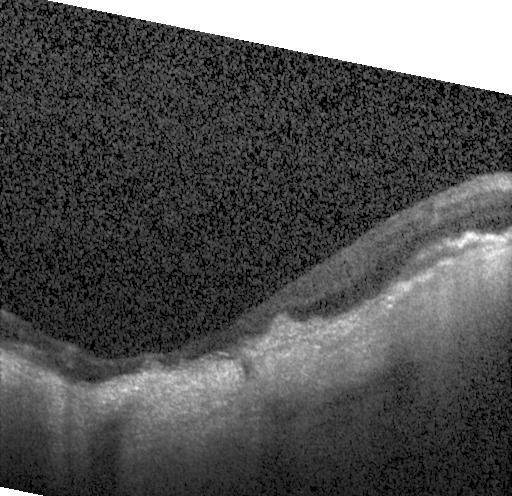

Impression: a choroidal neovascular membrane.